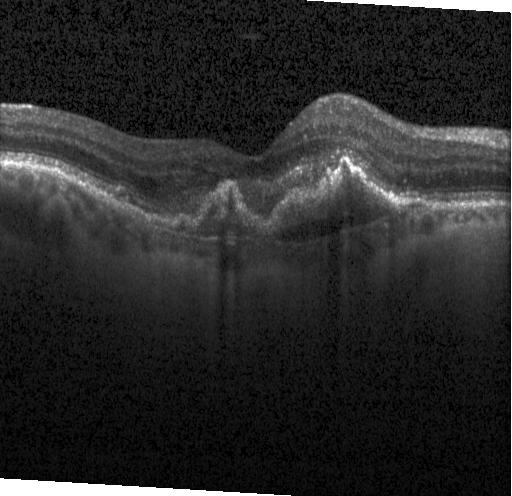
Horizontal scan through the fovea · instrument: Heidelberg Spectralis · spectral-domain optical coherence tomography · retinal OCT cross-section. Impression: a choroidal neovascular membrane.